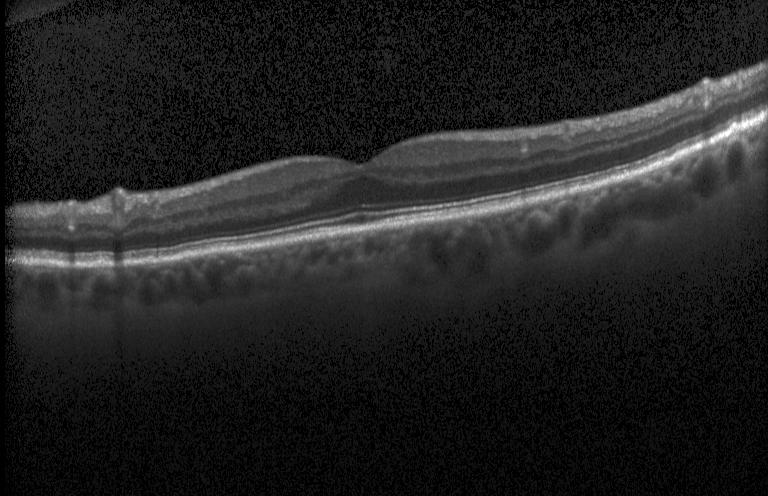

SD-OCT · Heidelberg Spectralis OCT system · optical coherence tomography scan. Impression: neither CNV, DME, nor drusen.